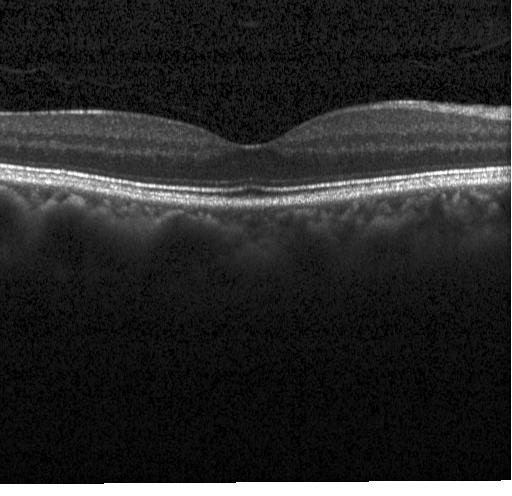

Optical coherence tomography scan.
Finding: no evidence of CNV, DME, or drusen.